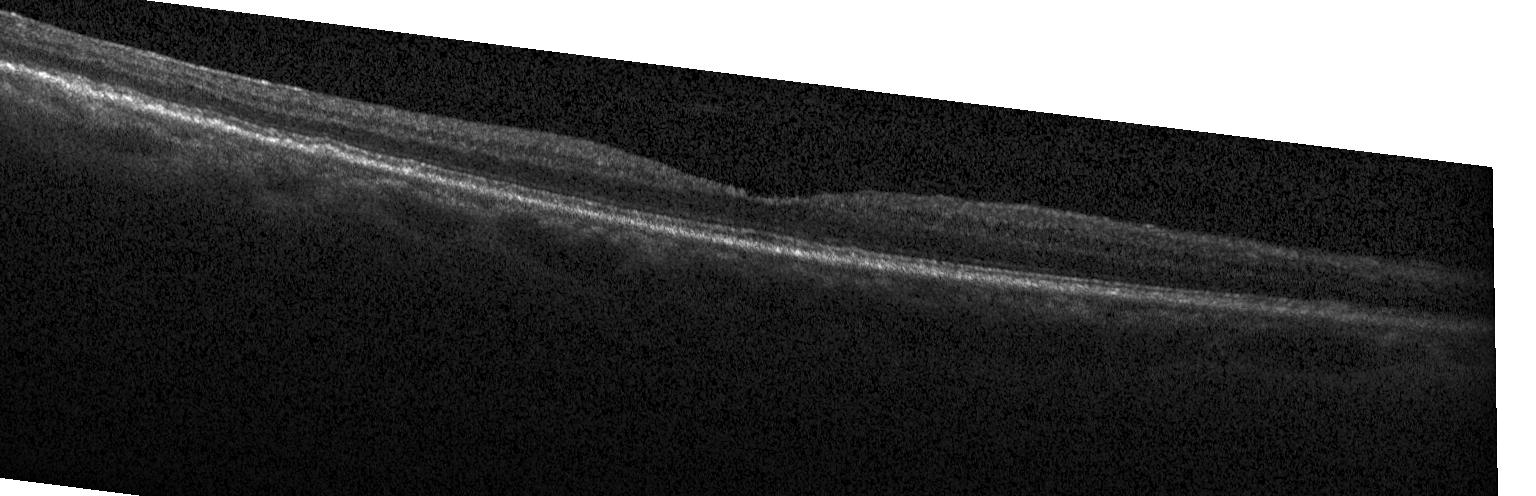

Spectral-domain optical coherence tomography · centered on the fovea · retinal OCT cross-section · Heidelberg Spectralis. Diagnosis: no choroidal neovascularization, no diabetic macular edema, and no drusen.